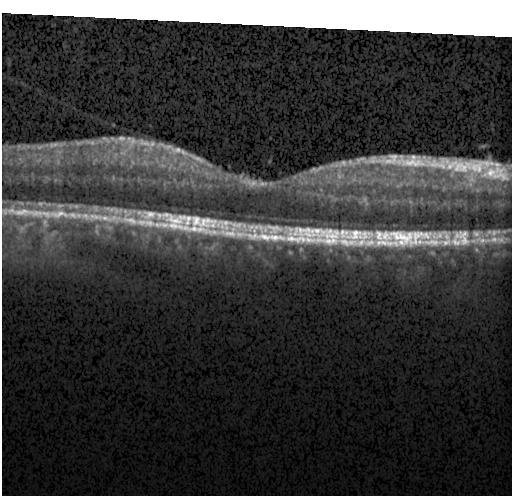
Fovea-centered, OCT line scan, spectral-domain OCT, acquired on a Heidelberg Spectralis — Macular OCT: neither CNV, DME, nor drusen.